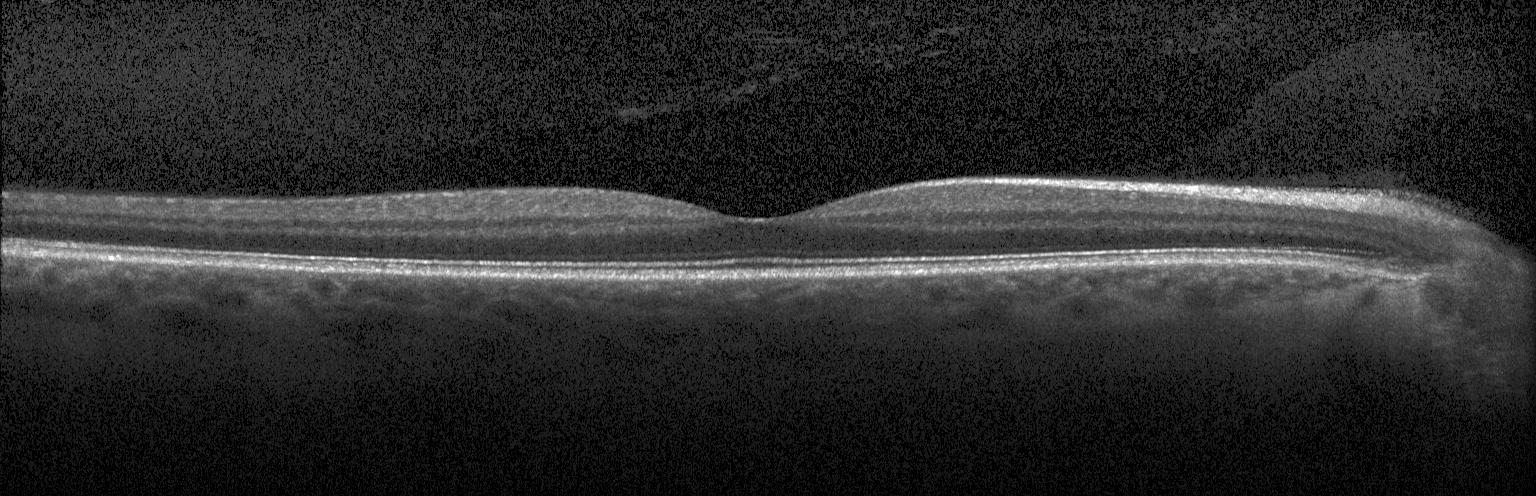

Diagnosis: no evidence of CNV, DME, or drusen.